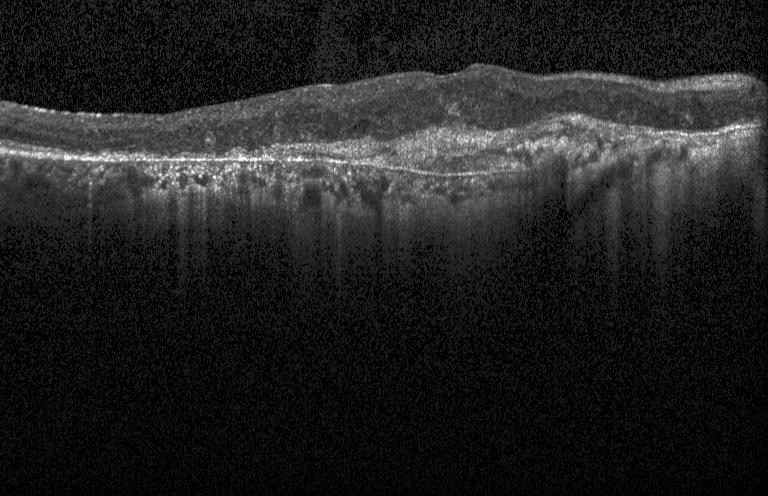 A choroidal neovascular membrane.